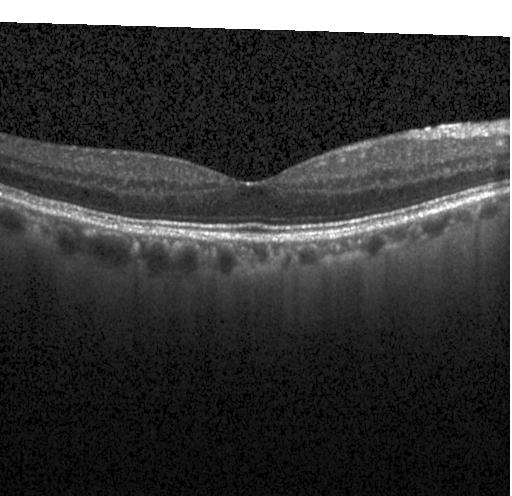

Spectral-domain OCT B-scan: neither CNV, DME, nor drusen.